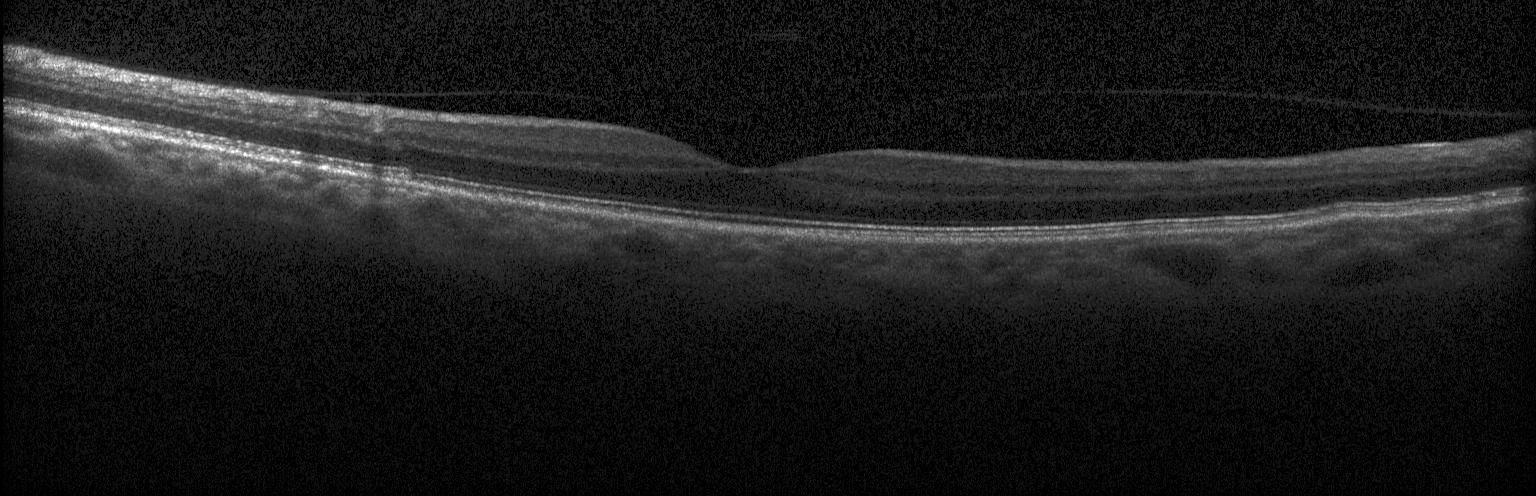
Assessment: neither choroidal neovascularization, diabetic macular edema, nor drusen.